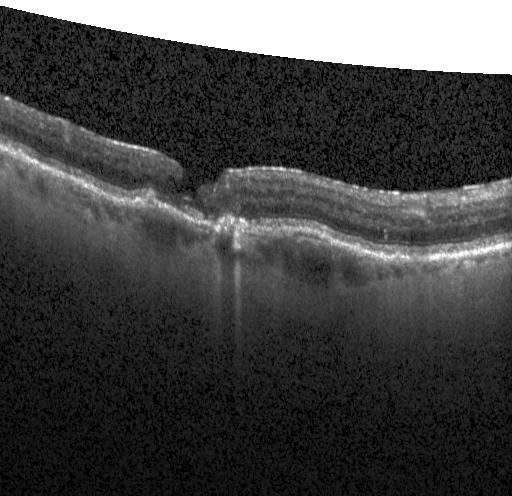

Optical coherence tomography scan
CNV.